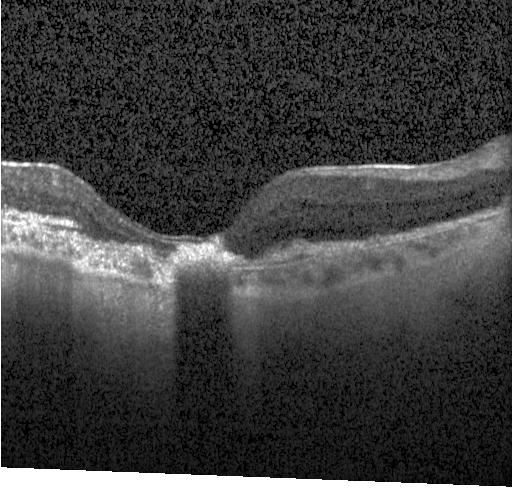 Acquired on a Heidelberg Spectralis; spectral-domain OCT; OCT line scan. A choroidal neovascular membrane.